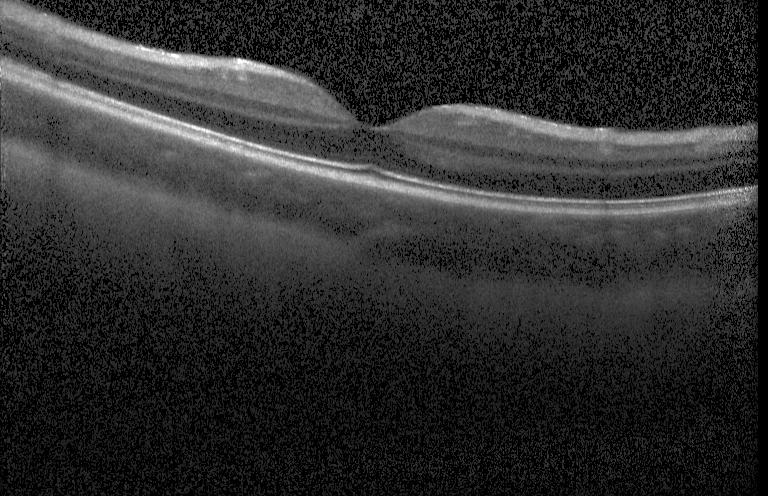

Horizontal scan through the fovea · Heidelberg Spectralis OCT system · OCT line scan · spectral-domain OCT — OCT finding: no evidence of CNV, DME, or drusen.